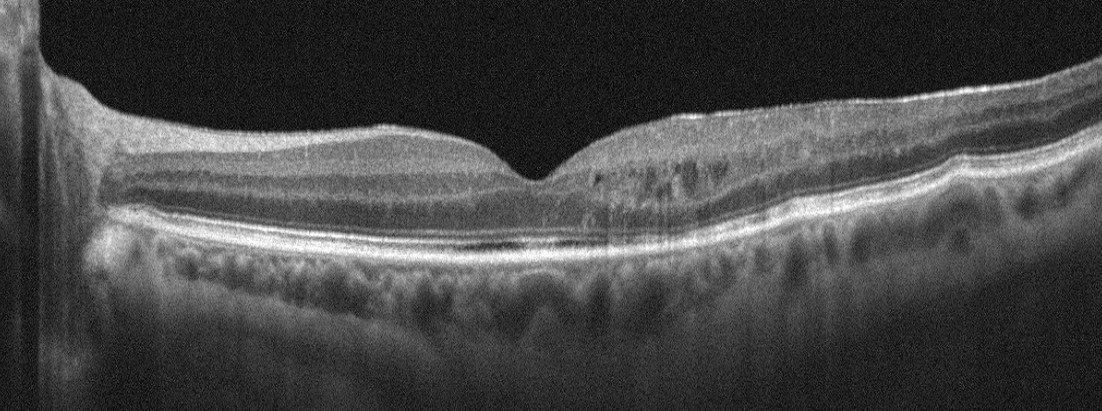 OCT finding: diabetic macular edema (DME).